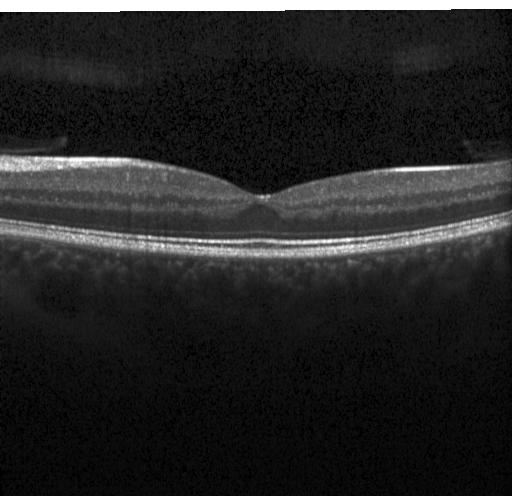
Finding: neither choroidal neovascularization, diabetic macular edema, nor drusen.